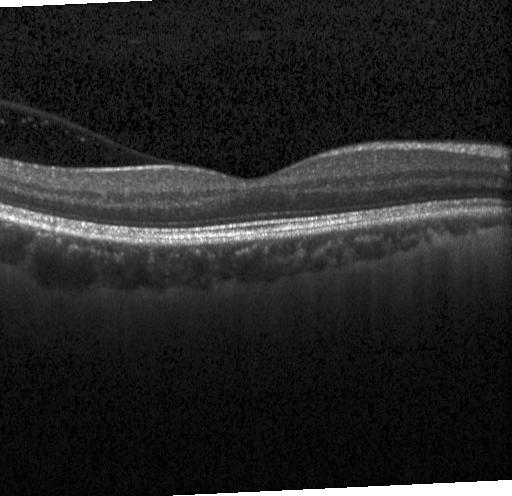 OCT line scan
Diagnosis: no CNV, no DME, and no drusen.